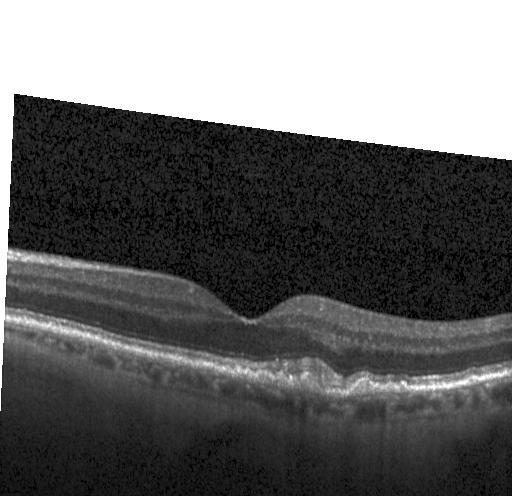
OCT finding: CNV.